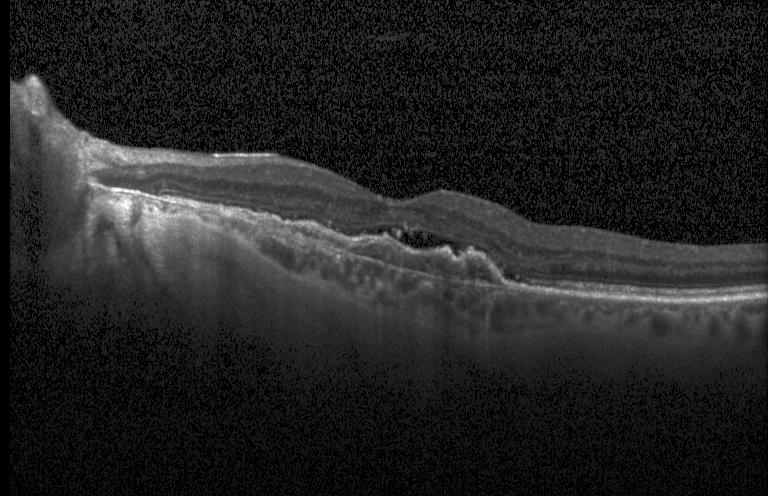

Spectral-domain OCT B-scan: CNV.